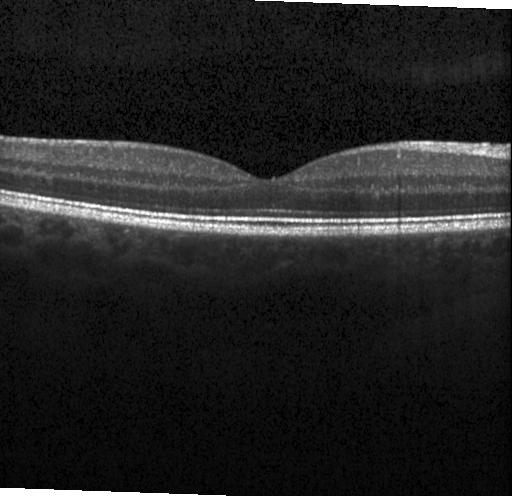

OCT scan showing neither choroidal neovascularization, diabetic macular edema, nor drusen.